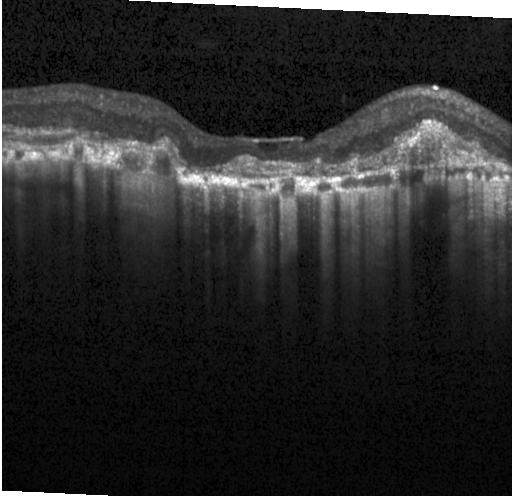 Spectral-domain optical coherence tomography. Macular scan. Acquired on a Heidelberg Spectralis. OCT line scan — Impression: a choroidal neovascular membrane.